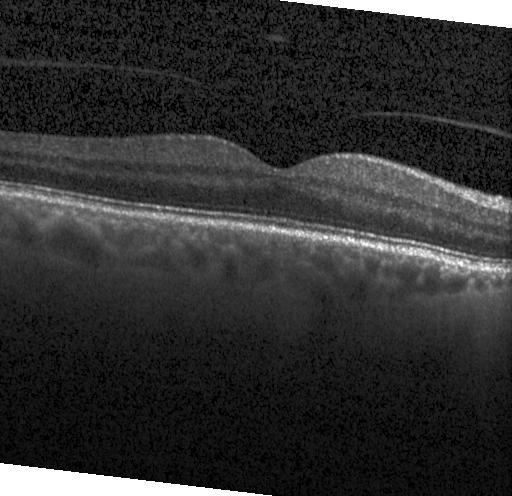 Optical coherence tomography B-scan — The scan shows no evidence of CNV, DME, or drusen.